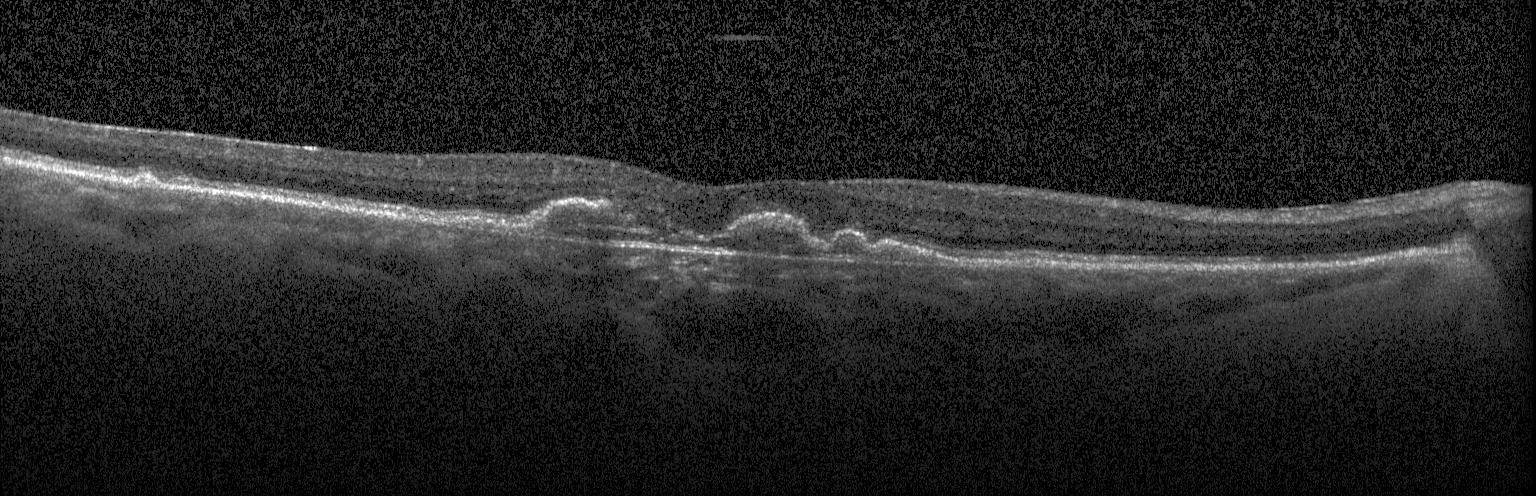 OCT line scan; Heidelberg Spectralis.
Assessment: a choroidal neovascular membrane.